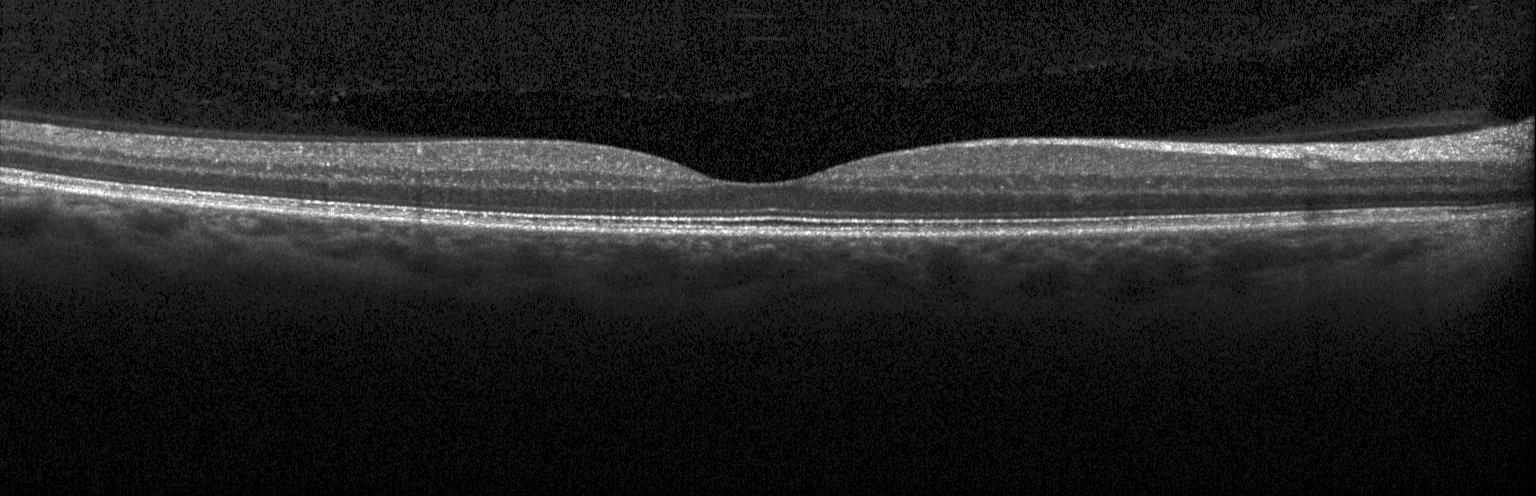

Spectral-domain optical coherence tomography, acquired on a Heidelberg Spectralis, OCT B-scan, macular scan. Impression: no choroidal neovascularization, no diabetic macular edema, and no drusen.